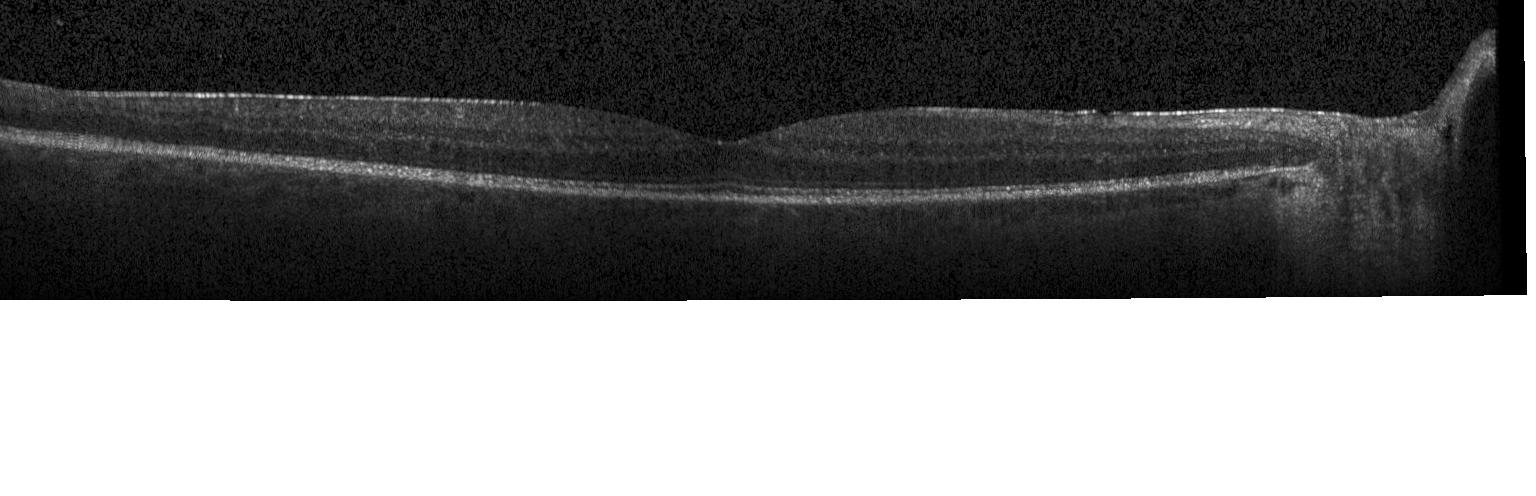 Optical coherence tomography B-scan. Through the macula. This B-scan demonstrates neither choroidal neovascularization, diabetic macular edema, nor drusen.